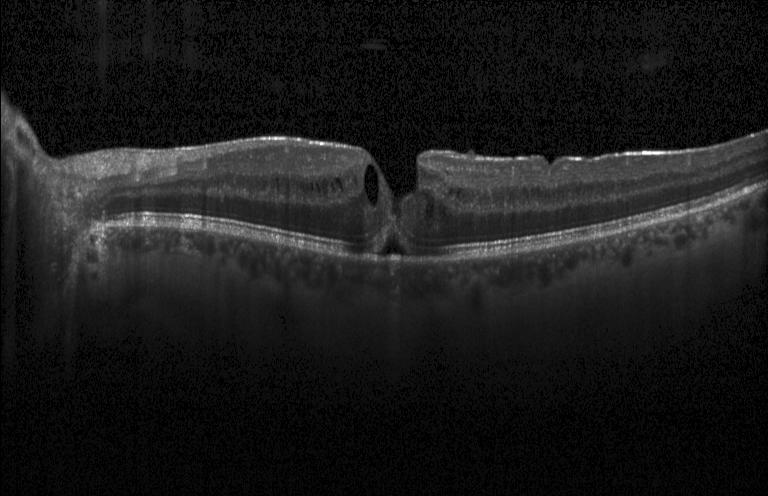

Optical coherence tomography B-scan. Macular scan. OCT finding: diabetic macular edema.